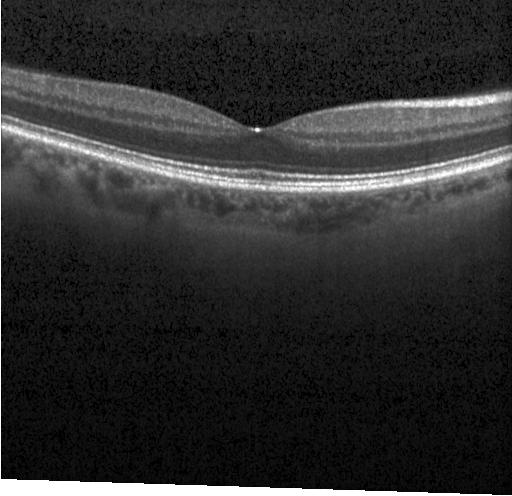
Optical coherence tomography scan. SD-OCT
Impression: neither choroidal neovascularization, diabetic macular edema, nor drusen.